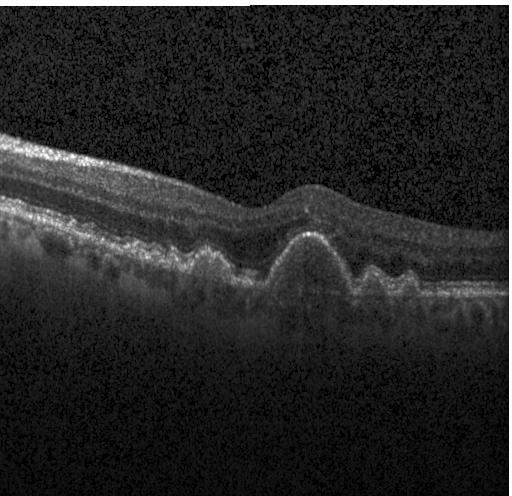
SD-OCT · instrument: Heidelberg Spectralis · optical coherence tomography B-scan · fovea-centered — OCT finding: sub-RPE drusenoid deposits.